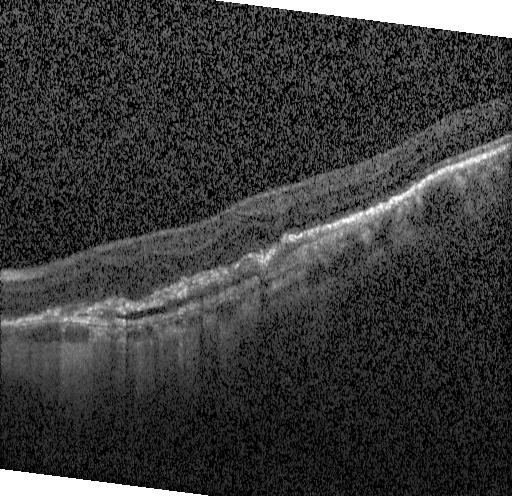 Impression: choroidal neovascularization.